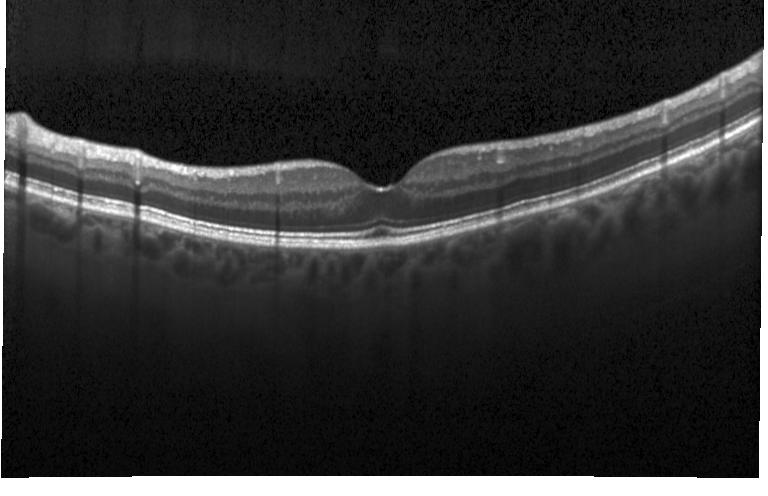

Optical coherence tomography scan. No evidence of choroidal neovascularization, diabetic macular edema, or drusen.